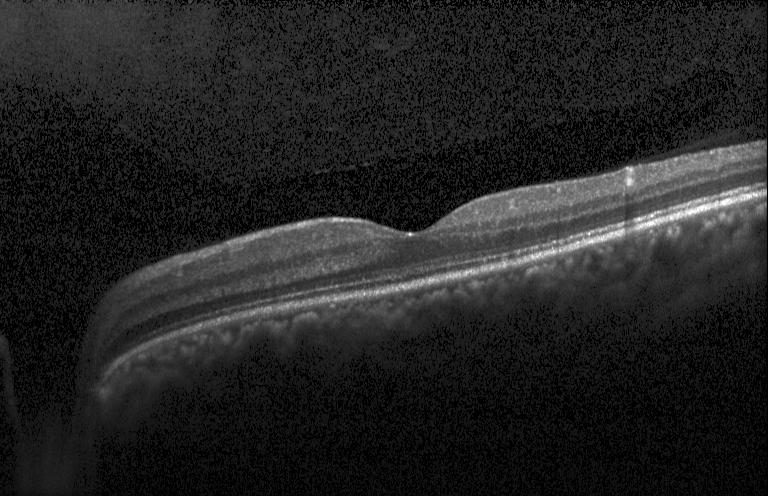 Centered on the fovea. OCT B-scan. Heidelberg Spectralis OCT system. Spectral-domain optical coherence tomography. This B-scan demonstrates no choroidal neovascularization, diabetic macular edema, or drusen.